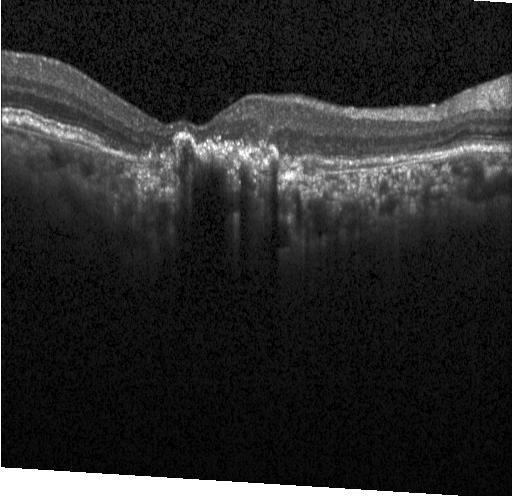
Retinal OCT cross-section showing choroidal neovascularization.